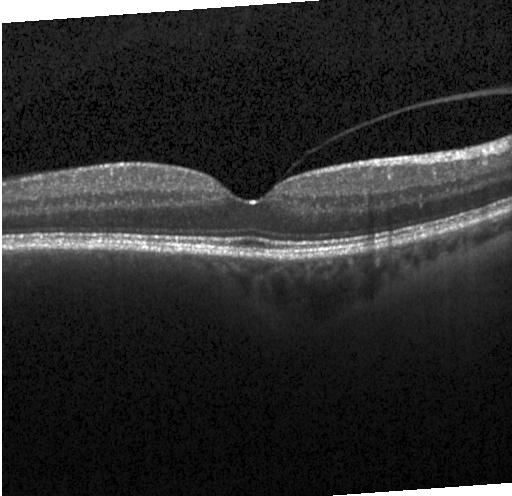

Spectral-domain OCT. OCT line scan
Finding: no evidence of choroidal neovascularization, diabetic macular edema, or drusen.